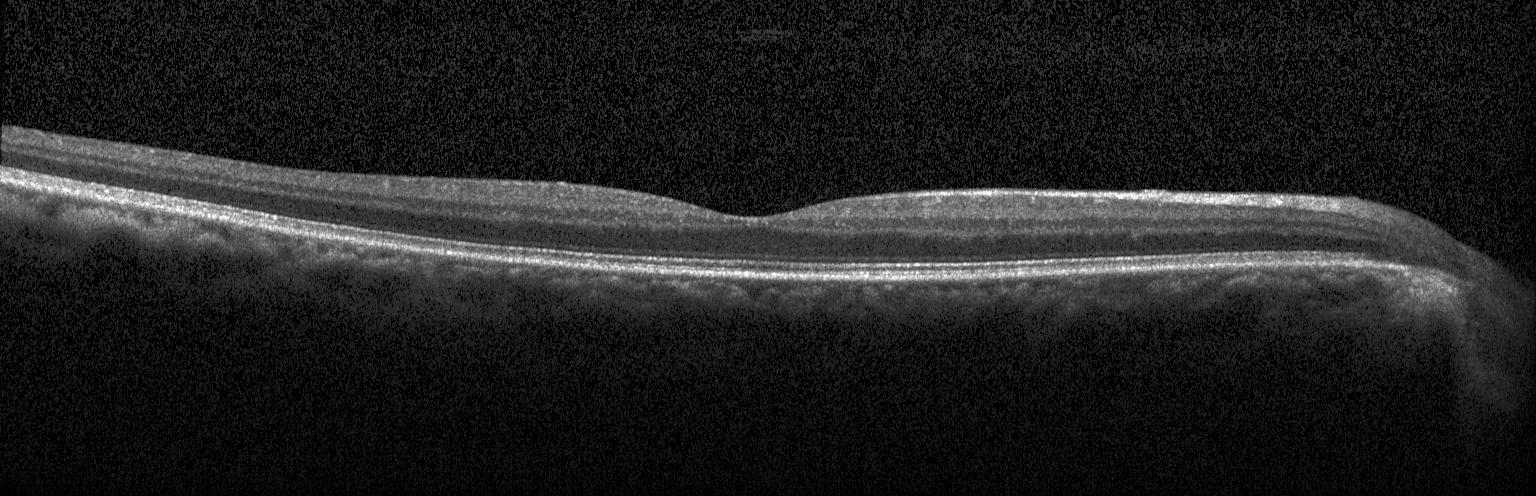

No evidence of choroidal neovascularization, diabetic macular edema, or drusen.